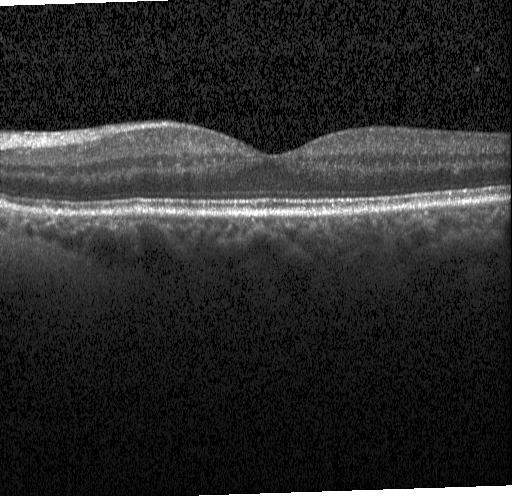

Spectral-domain OCT B-scan: neither choroidal neovascularization, diabetic macular edema, nor drusen.